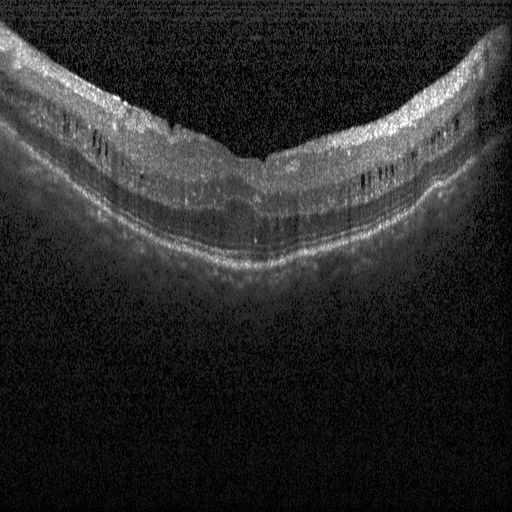

Heidelberg Spectralis OCT system, retinal OCT B-scan — The scan shows diabetic macular edema (DME).